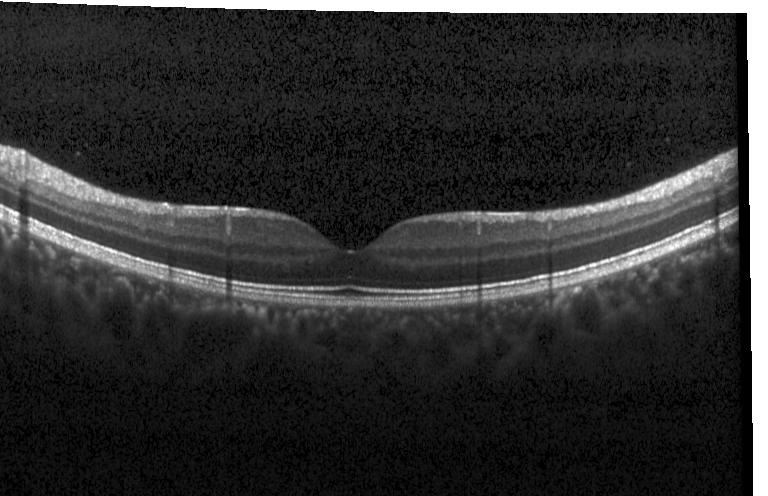 Spectral-domain optical coherence tomography. OCT line scan. Acquired on a Heidelberg Spectralis
Assessment: neither choroidal neovascularization, diabetic macular edema, nor drusen.